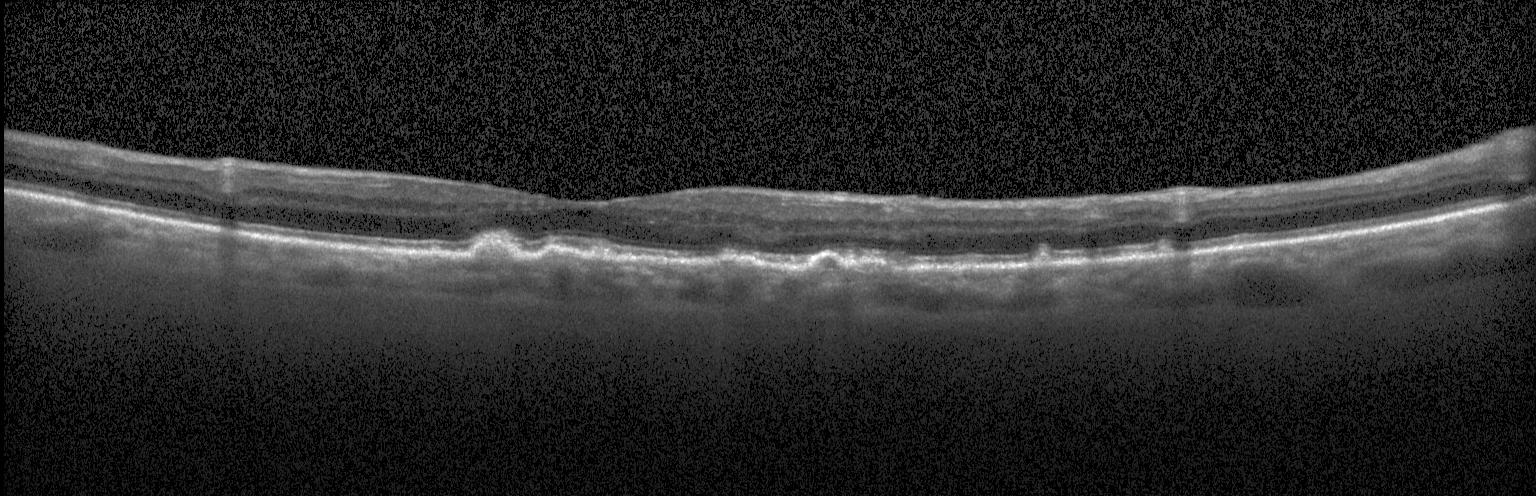

The scan shows multiple drusen.